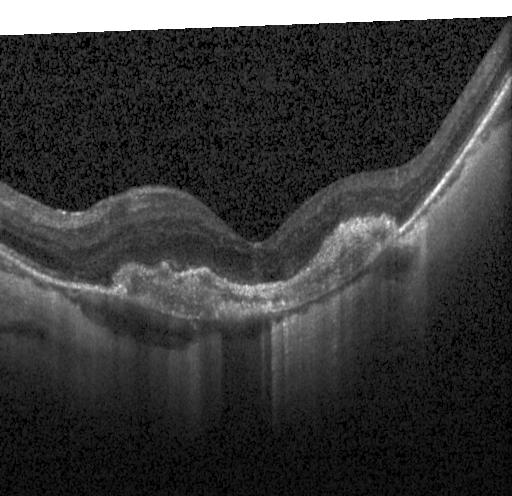

Diagnosis: a choroidal neovascular membrane.